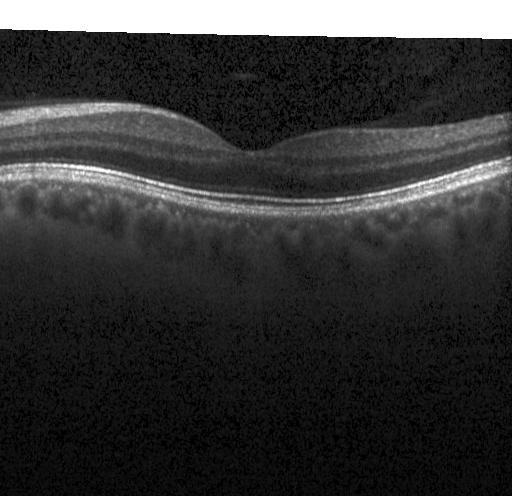

Horizontal scan through the fovea; OCT line scan — Neither choroidal neovascularization, diabetic macular edema, nor drusen.